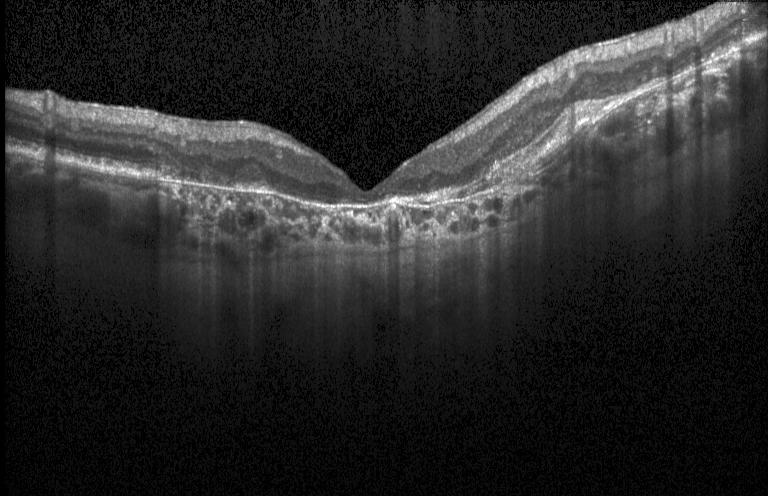

The scan shows a choroidal neovascular membrane.